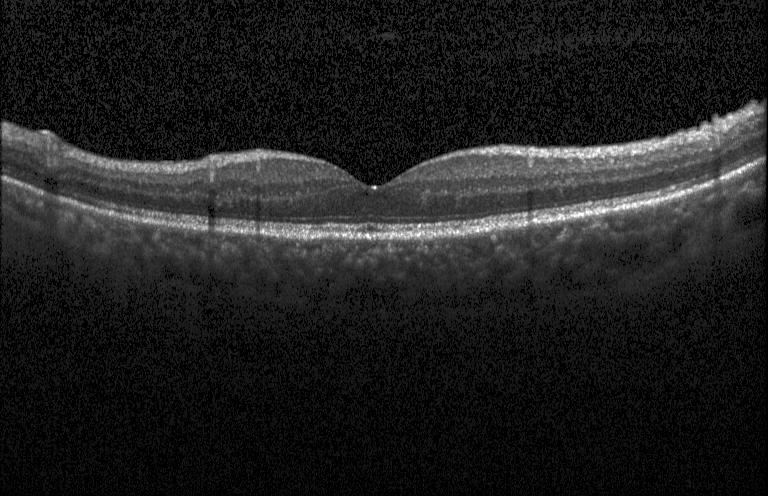
Heidelberg Spectralis, through the macula, retinal OCT cross-section, spectral-domain optical coherence tomography
Assessment: no choroidal neovascularization, no diabetic macular edema, and no drusen.